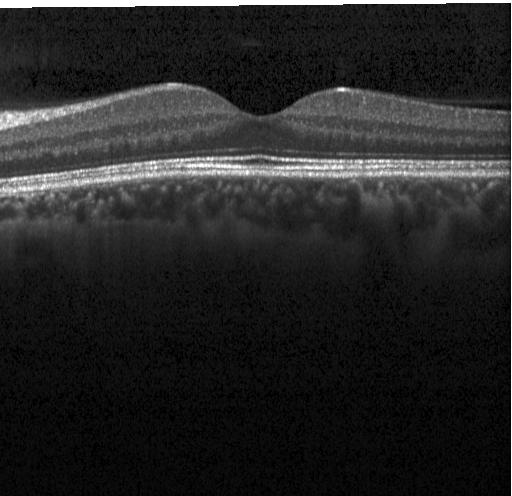
Finding: neither choroidal neovascularization, diabetic macular edema, nor drusen.